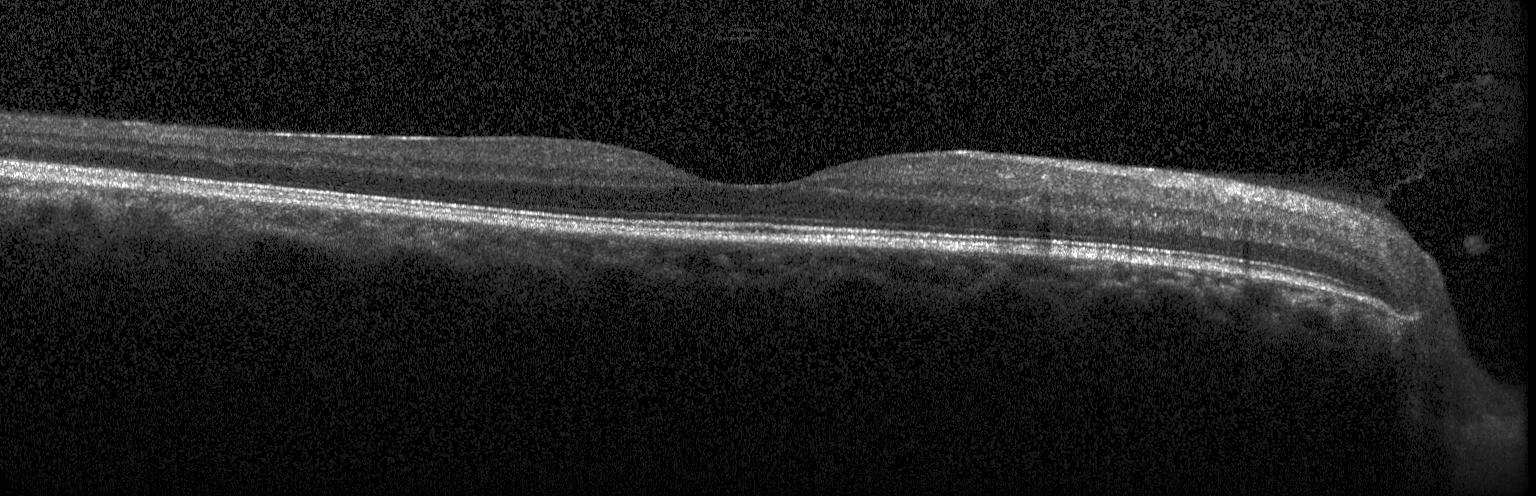
Spectral-domain OCT B-scan: no CNV, no DME, and no drusen.